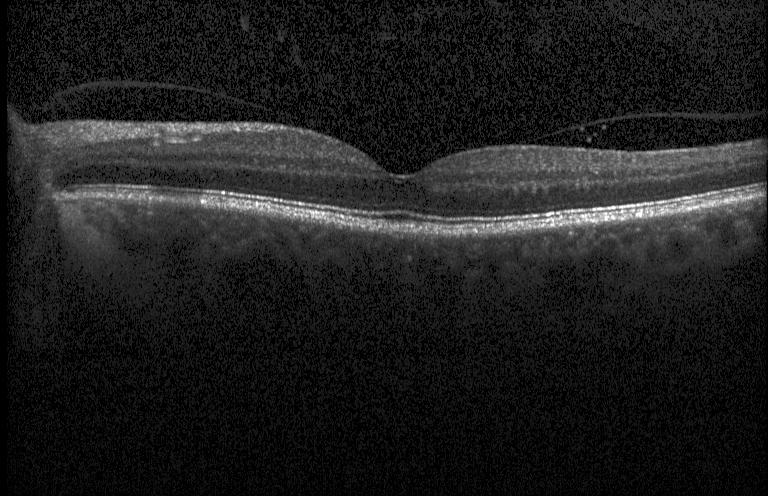
Optical coherence tomography scan.
Finding: neither choroidal neovascularization, diabetic macular edema, nor drusen.